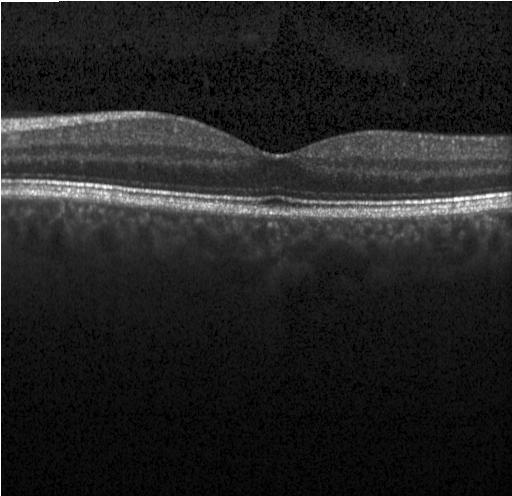 Macular OCT: no CNV, DME, or drusen.